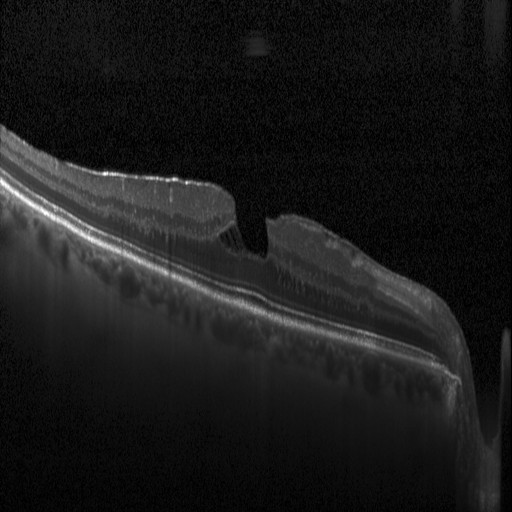
Optical coherence tomography B-scan · fovea-centered · acquired on a Heidelberg Spectralis · spectral-domain OCT.
The scan shows diabetic macular edema (DME).